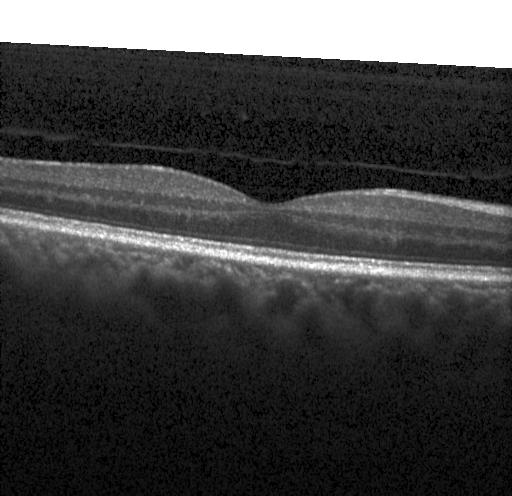
Macular OCT demonstrating no choroidal neovascularization, diabetic macular edema, or drusen.